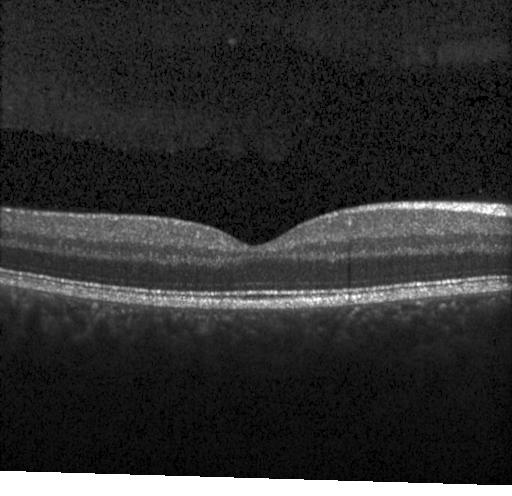
Spectral-domain optical coherence tomography · optical coherence tomography scan
Neither choroidal neovascularization, diabetic macular edema, nor drusen.